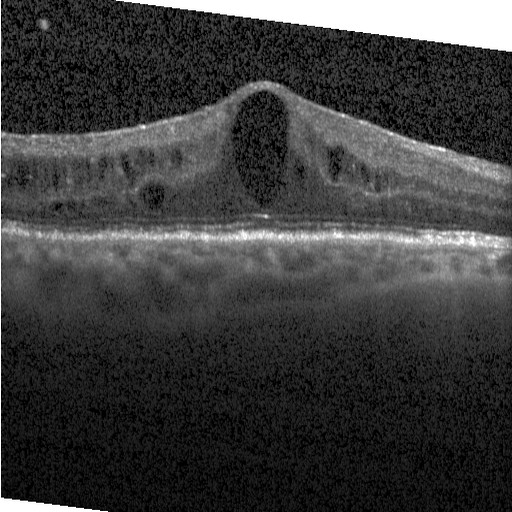

Impression: diabetic macular edema.